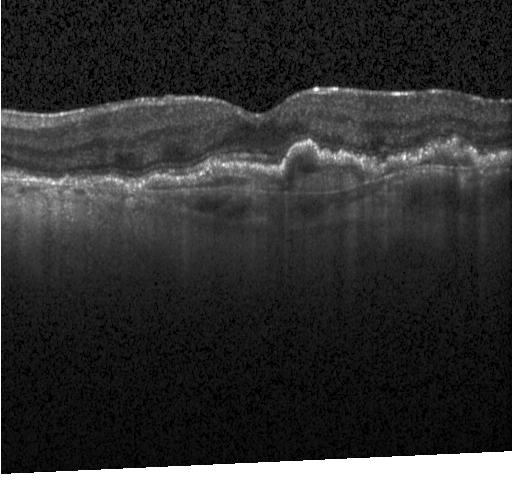
Diagnosis: a choroidal neovascular membrane.